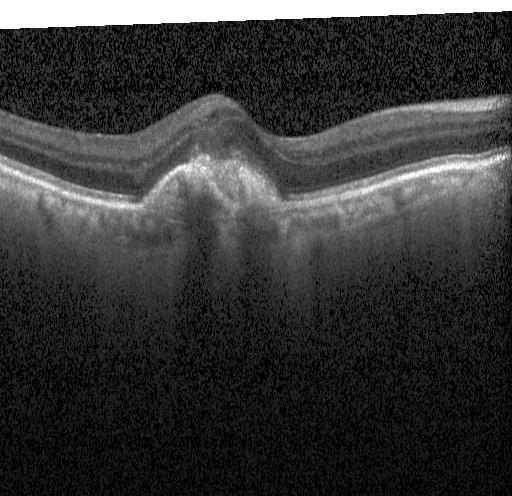
Impression: a choroidal neovascular membrane.